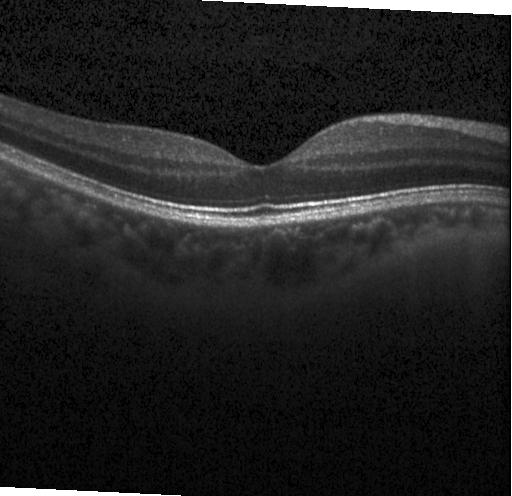 Macular scan; OCT line scan — OCT finding: no CNV, no DME, and no drusen.